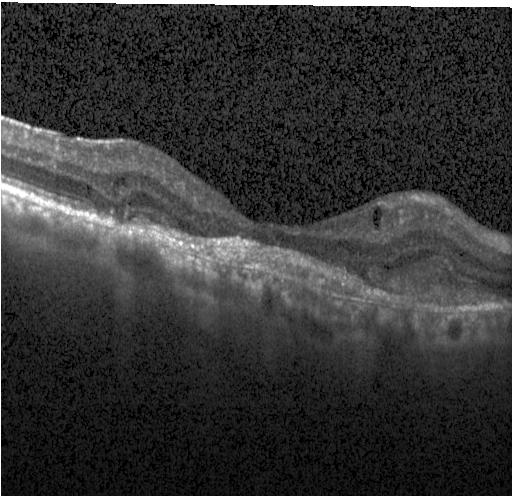

Optical coherence tomography B-scan, through the macula.
Impression: CNV.